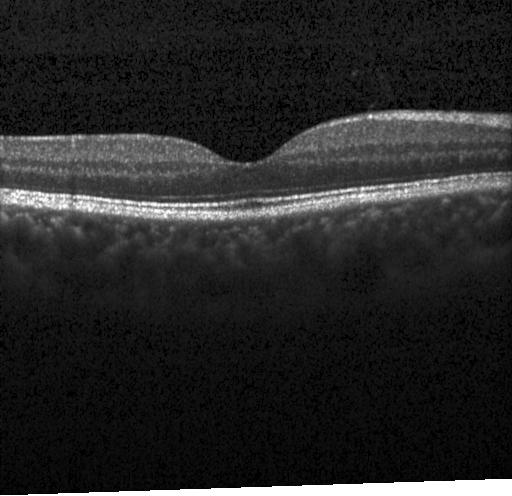
OCT B-scan showing no evidence of choroidal neovascularization, diabetic macular edema, or drusen.